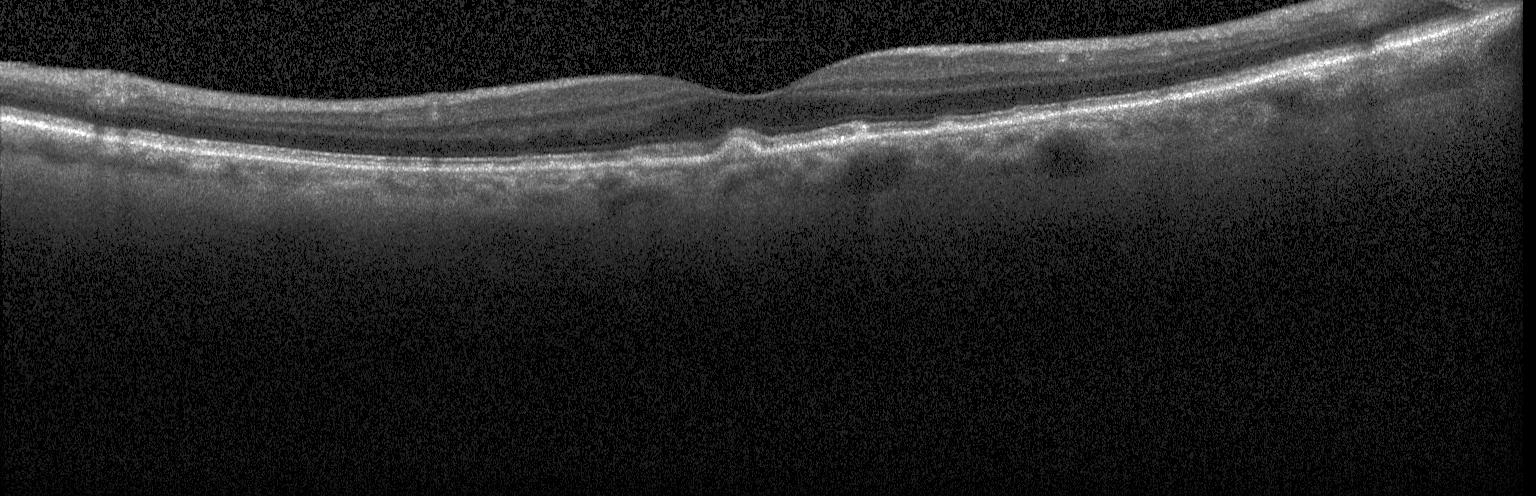 The scan shows sub-RPE drusenoid deposits.